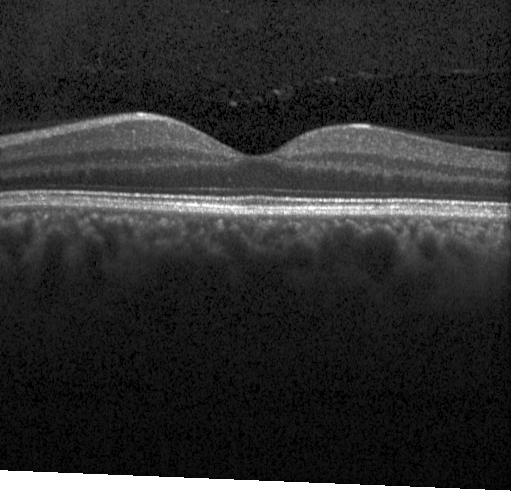
Fovea-centered. Retinal OCT cross-section. SD-OCT. Heidelberg Spectralis OCT system
The scan shows no choroidal neovascularization, no diabetic macular edema, and no drusen.